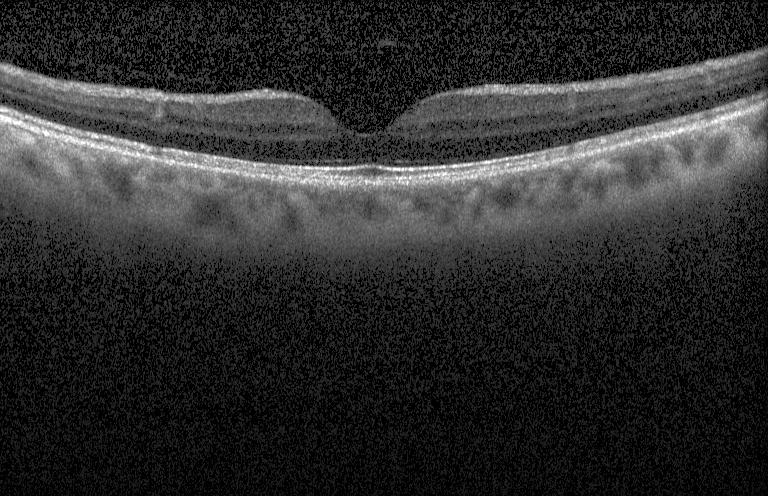 Optical coherence tomography B-scan
OCT finding: neither choroidal neovascularization, diabetic macular edema, nor drusen.